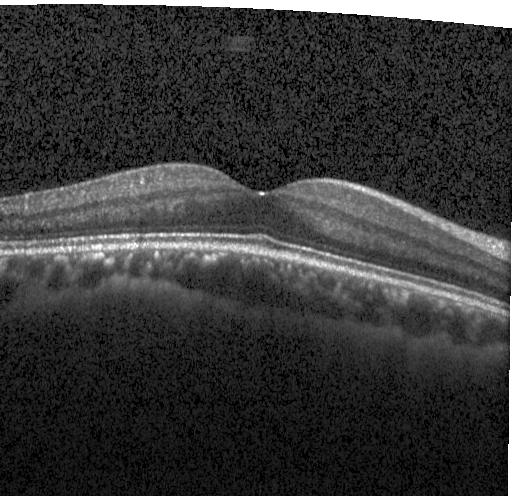 Impression: no choroidal neovascularization, no diabetic macular edema, and no drusen.